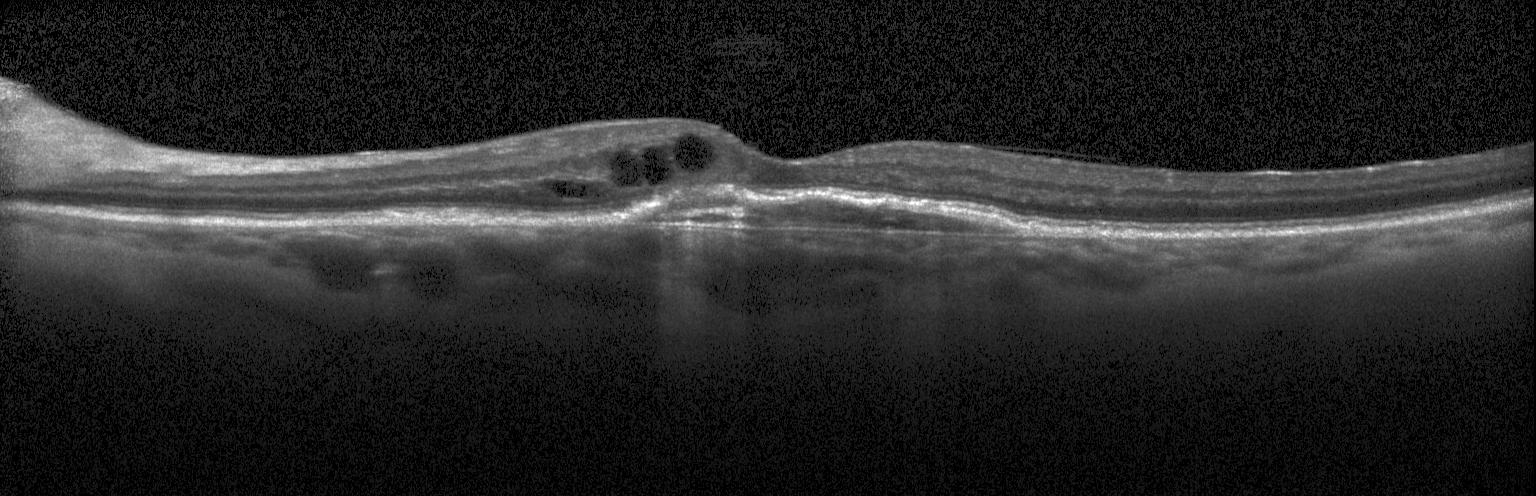

This B-scan demonstrates a choroidal neovascular membrane.